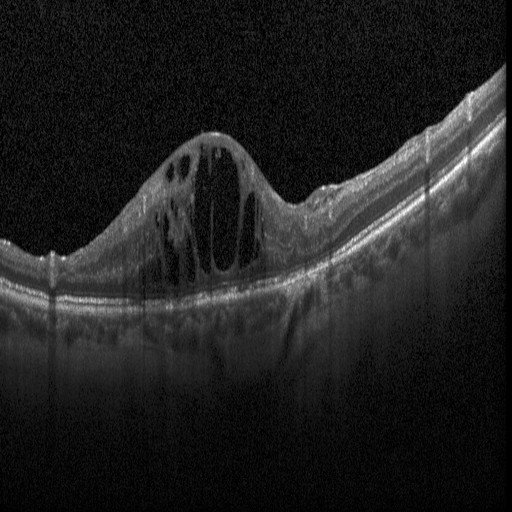 Macular OCT demonstrating DME.